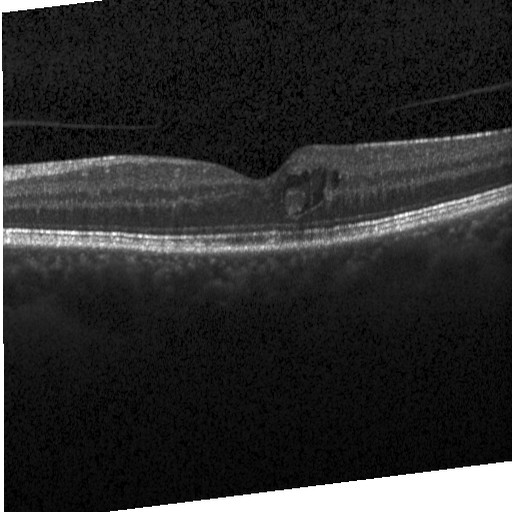
Macular scan, spectral-domain OCT, optical coherence tomography scan.
Impression: DME.